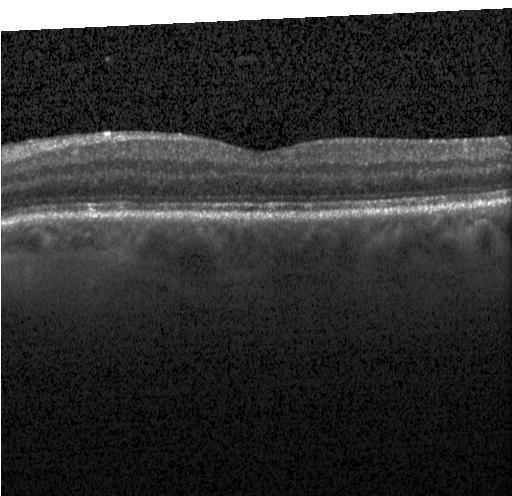 Finding: no choroidal neovascularization, diabetic macular edema, or drusen.